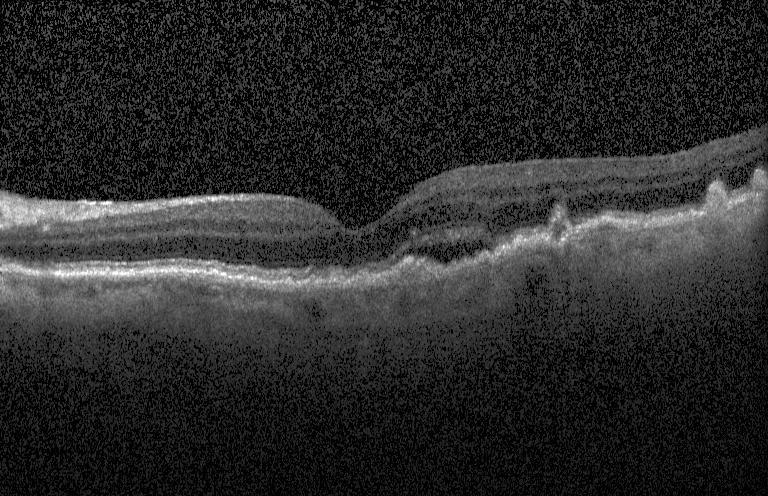
OCT B-scan showing CNV.